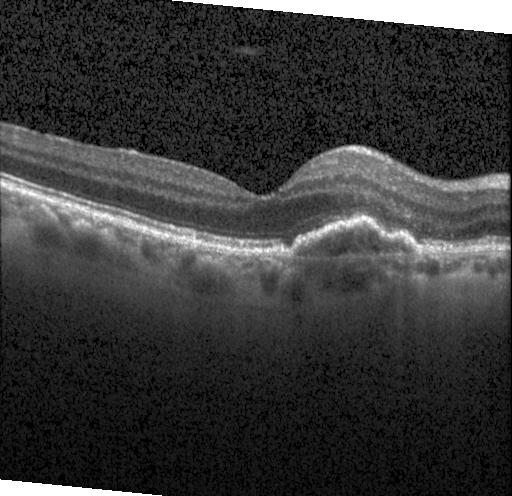
OCT finding: CNV.